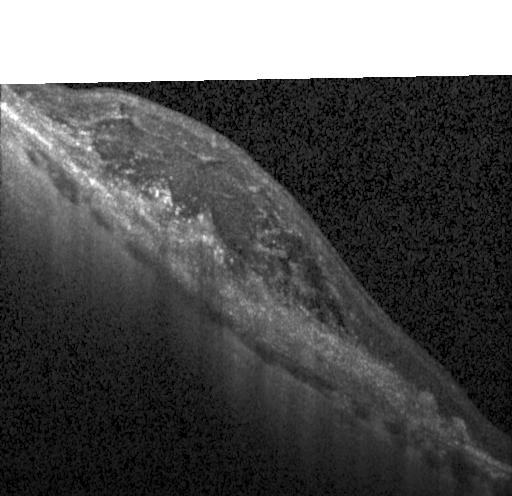
Centered on the fovea. Optical coherence tomography B-scan. Acquired on a Heidelberg Spectralis. SD-OCT
Diagnosis: choroidal neovascularization.